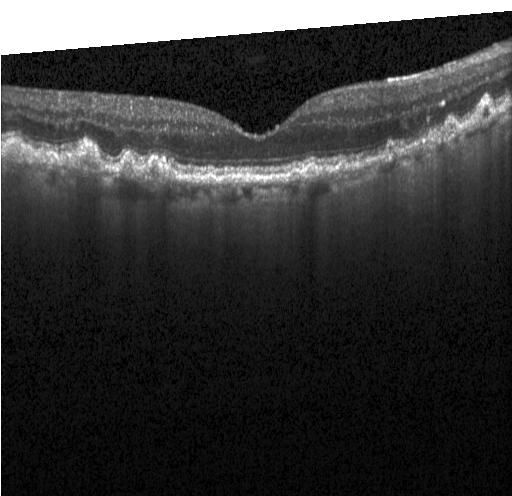 Retinal OCT cross-section; spectral-domain optical coherence tomography; through the macula; Heidelberg Spectralis.
Impression: sub-RPE drusenoid deposits.